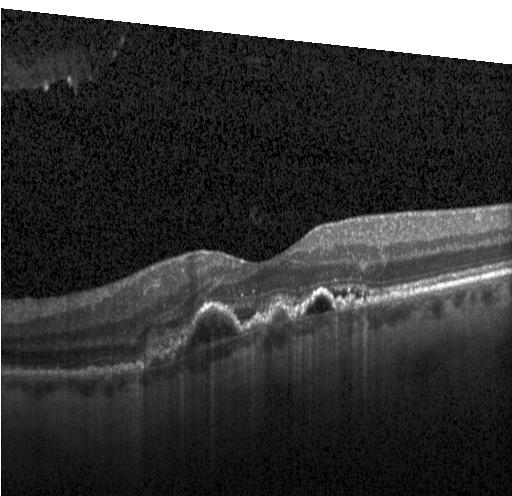
Horizontal scan through the fovea · spectral-domain OCT · retinal OCT B-scan — Diagnosis: choroidal neovascularization.